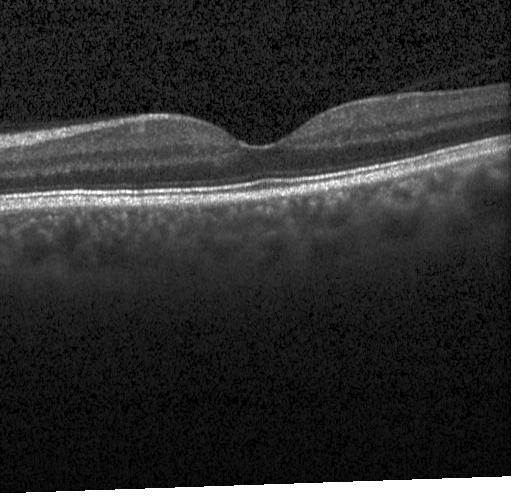

Retinal OCT cross-section showing no choroidal neovascularization, diabetic macular edema, or drusen.